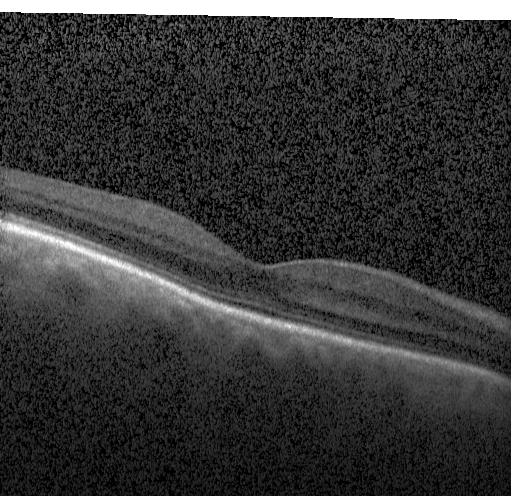
Macular scan. Spectral-domain optical coherence tomography. Retinal OCT cross-section
The scan shows no evidence of choroidal neovascularization, diabetic macular edema, or drusen.